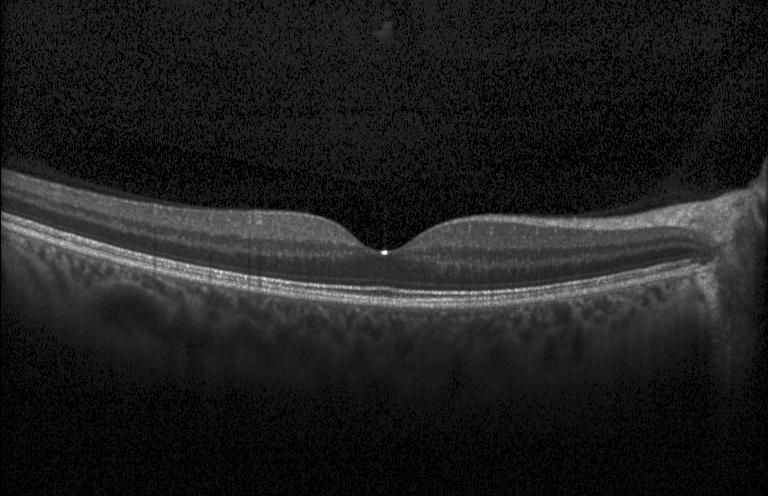

Retinal OCT B-scan
No evidence of choroidal neovascularization, diabetic macular edema, or drusen.